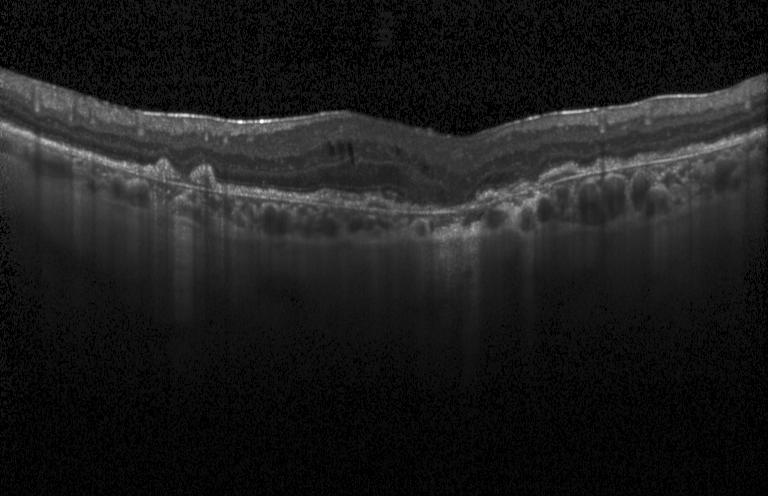

Dx: a choroidal neovascular membrane.